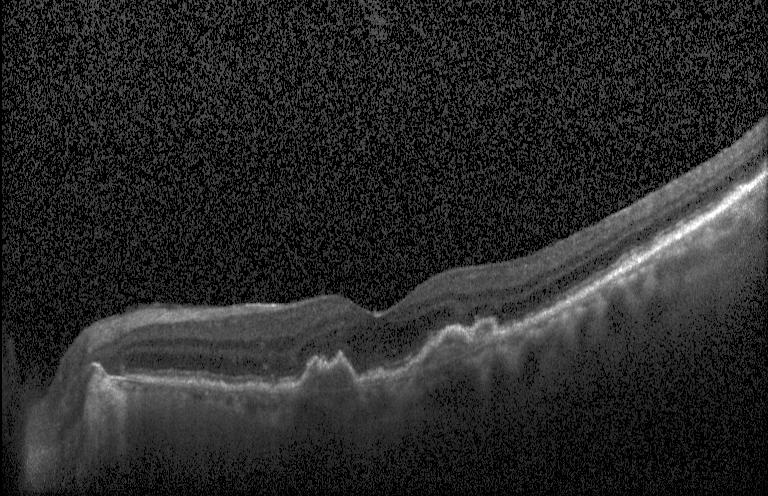 Spectral-domain OCT. OCT line scan. Macular scan. Acquired on a Heidelberg Spectralis
Dx: a choroidal neovascular membrane.